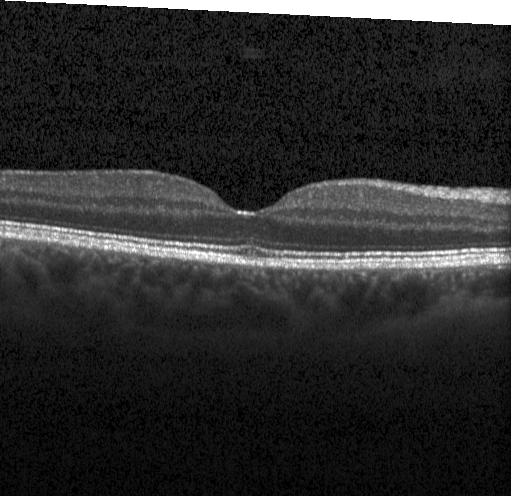
Instrument: Heidelberg Spectralis. Spectral-domain OCT. Retinal OCT B-scan. Through the macula
Diagnosis: no choroidal neovascularization, no diabetic macular edema, and no drusen.